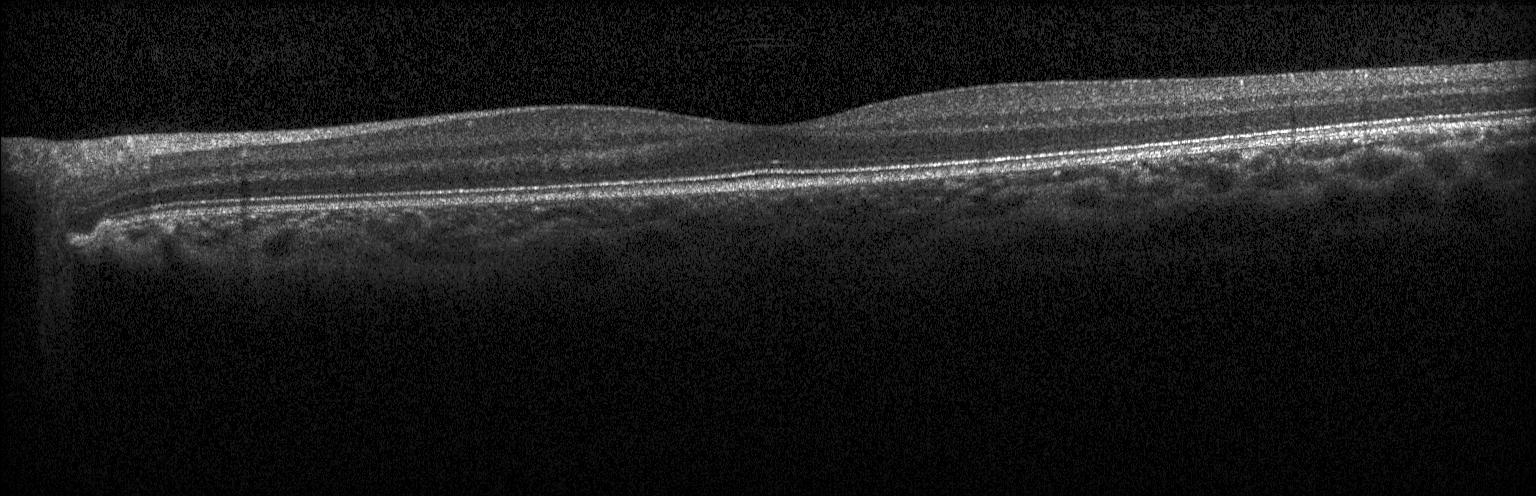

OCT B-scan showing no evidence of choroidal neovascularization, diabetic macular edema, or drusen.